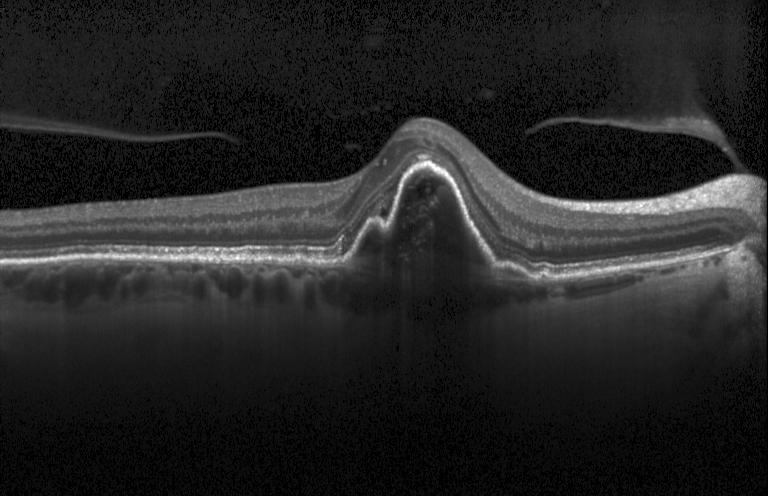
This B-scan demonstrates a choroidal neovascular membrane.